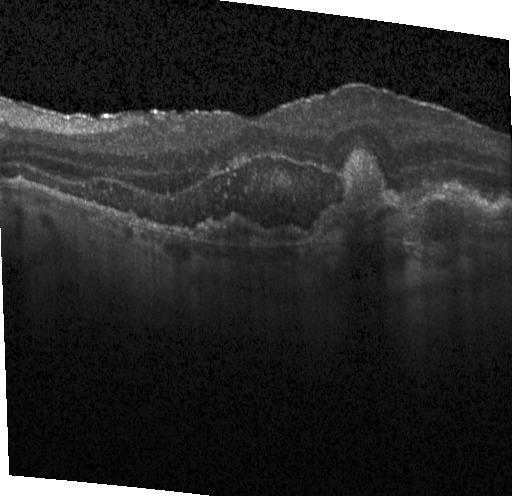 Centered on the fovea. Optical coherence tomography B-scan. Spectral-domain OCT. Acquired on a Heidelberg Spectralis — Diagnosis: a choroidal neovascular membrane.